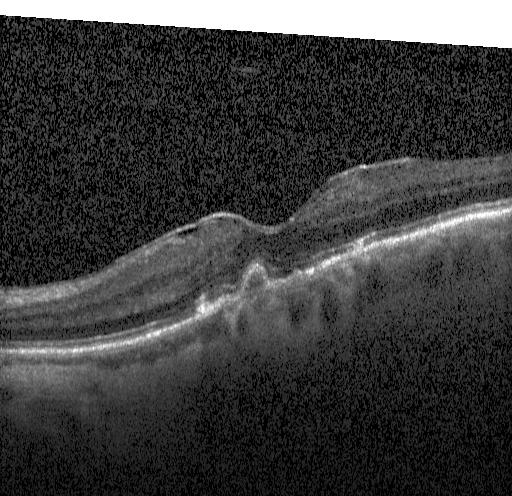

Impression: drusen.